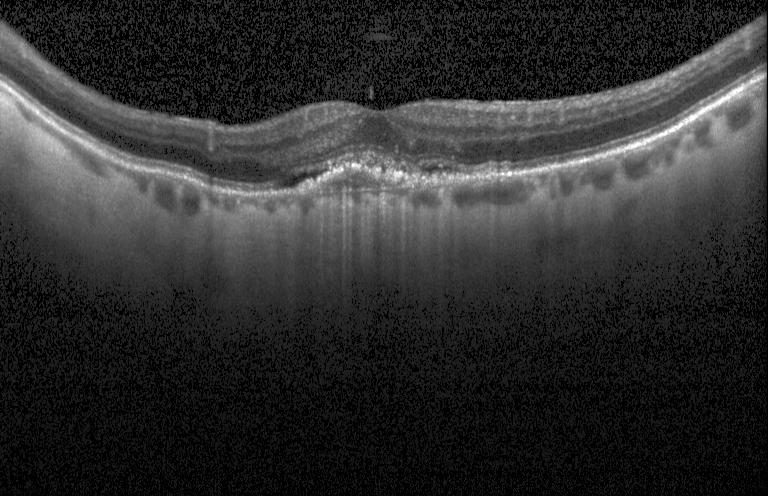
Retinal OCT B-scan; Heidelberg Spectralis OCT system. Diagnosis: a choroidal neovascular membrane.